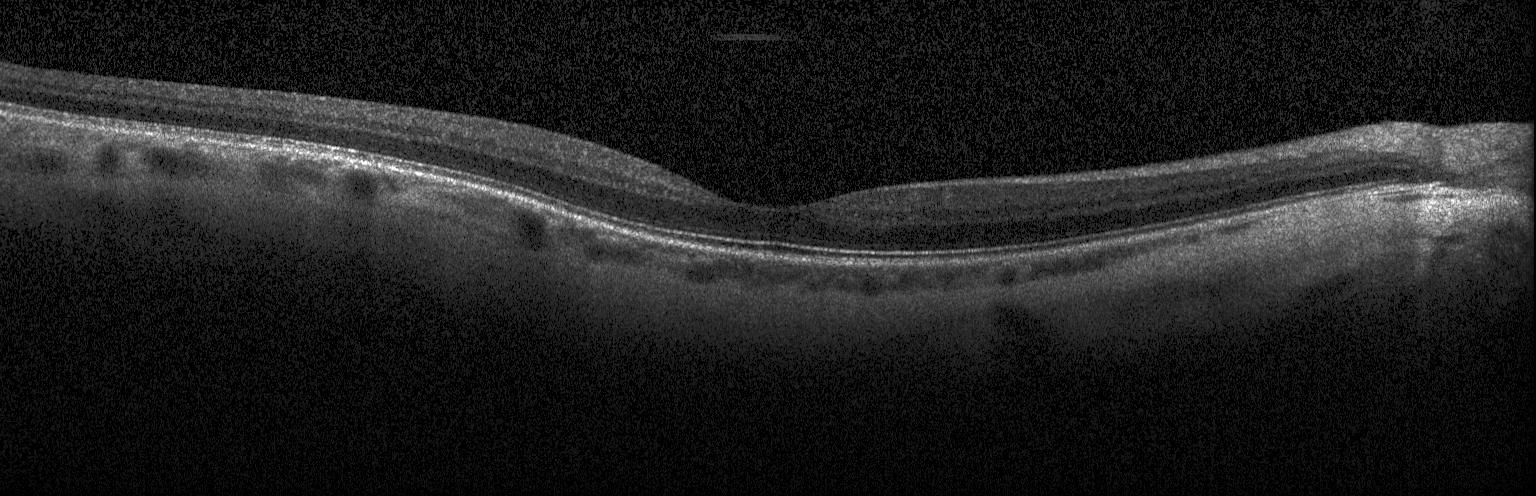
Fovea-centered, instrument: Heidelberg Spectralis, OCT B-scan, spectral-domain optical coherence tomography
Diagnosis: neither choroidal neovascularization, diabetic macular edema, nor drusen.